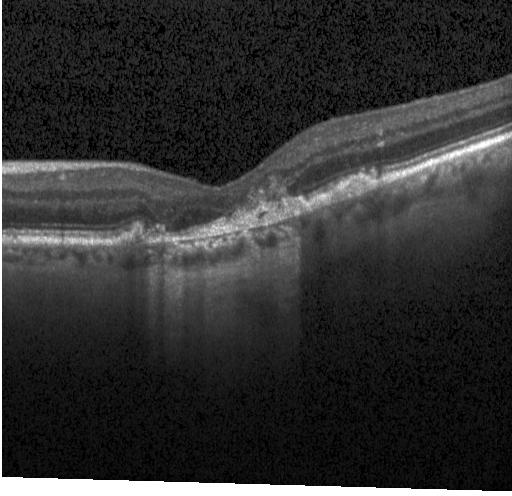
Retinal OCT B-scan; SD-OCT; horizontal scan through the fovea; acquired on a Heidelberg Spectralis — Dx: a choroidal neovascular membrane.